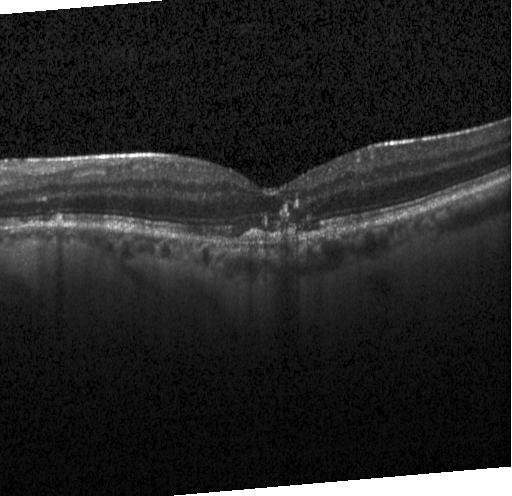
OCT line scan.
Dx: choroidal neovascularization (CNV).